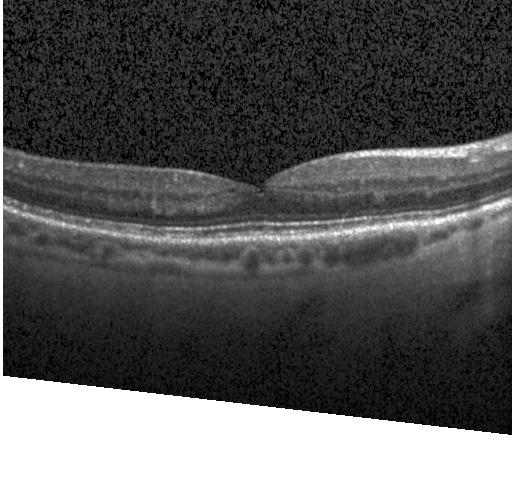

Spectral-domain OCT · retinal OCT B-scan — Finding: no choroidal neovascularization, diabetic macular edema, or drusen.